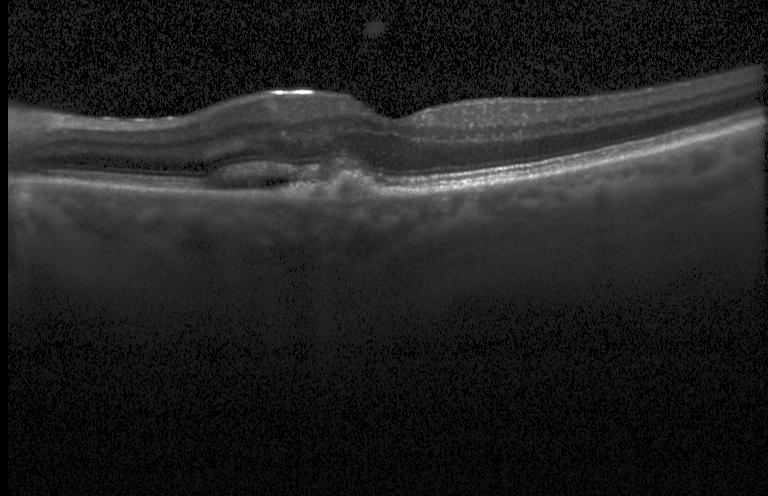 Spectral-domain OCT B-scan: choroidal neovascularization (CNV).